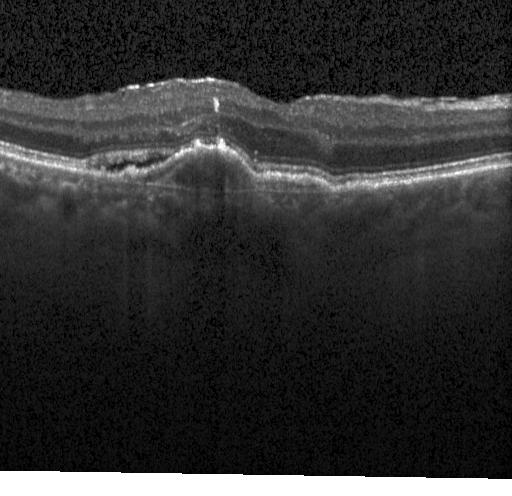 Retinal OCT cross-section showing a choroidal neovascular membrane.